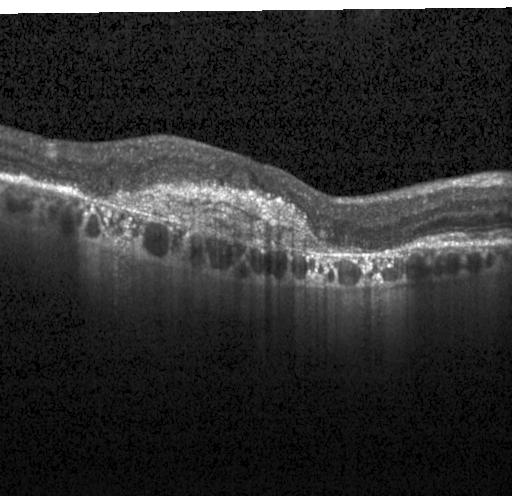

Spectral-domain OCT B-scan: a choroidal neovascular membrane.